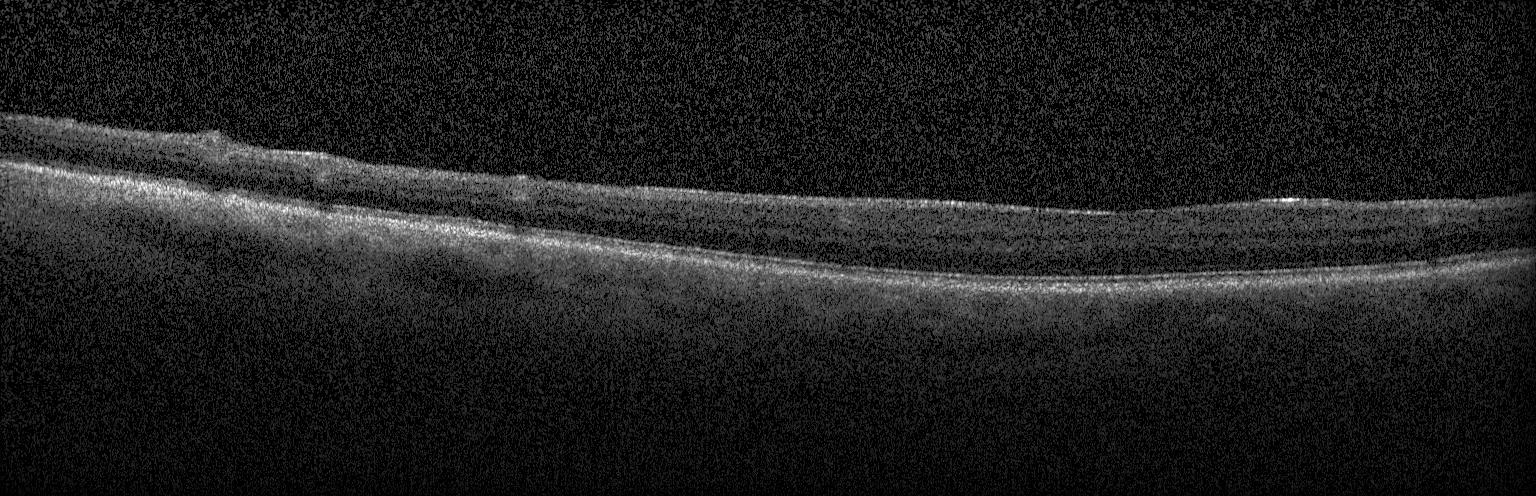 Impression: no evidence of choroidal neovascularization, diabetic macular edema, or drusen.